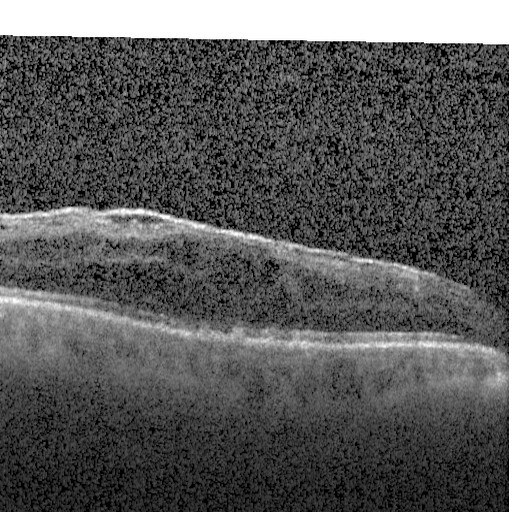

Assessment: diabetic macular edema (DME).